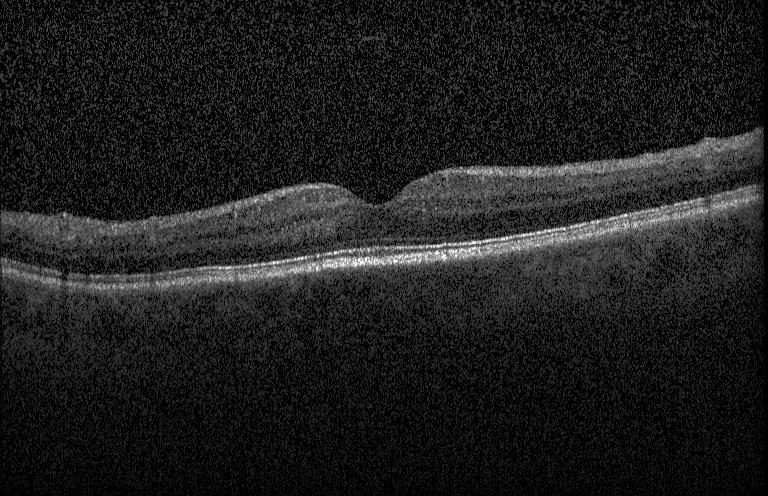
This B-scan demonstrates no CNV, no DME, and no drusen.